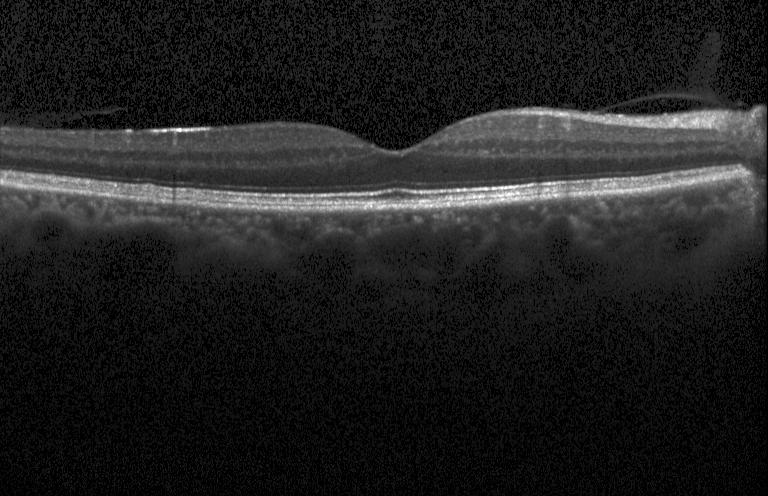
Macular OCT: no CNV, no DME, and no drusen.